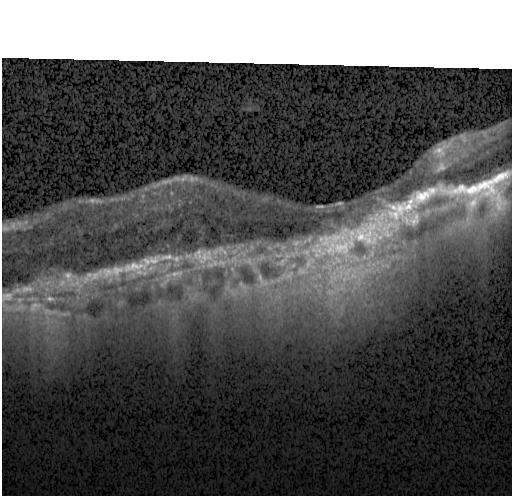
OCT line scan. Heidelberg Spectralis OCT system. Macular scan. Spectral-domain optical coherence tomography — Diagnosis: choroidal neovascularization.